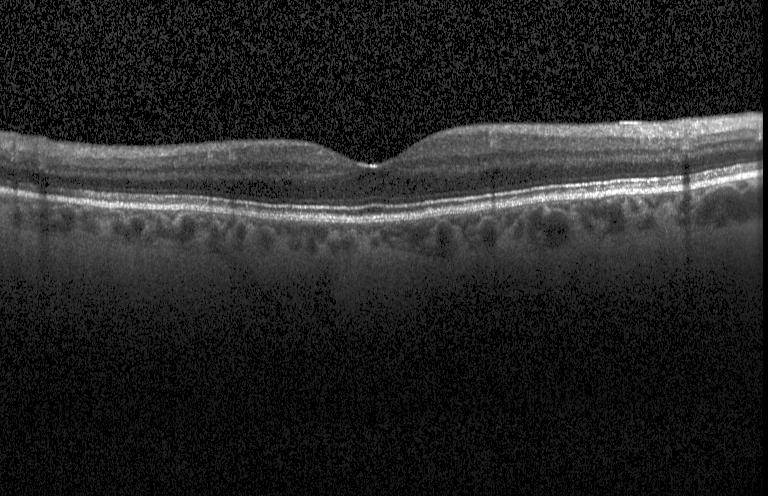 No choroidal neovascularization, no diabetic macular edema, and no drusen.